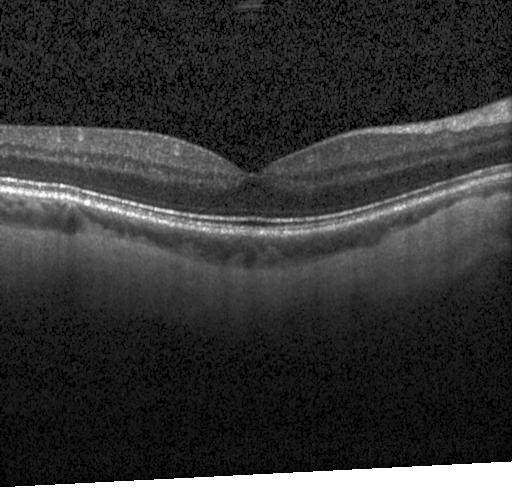 OCT B-scan
The scan shows no choroidal neovascularization, diabetic macular edema, or drusen.